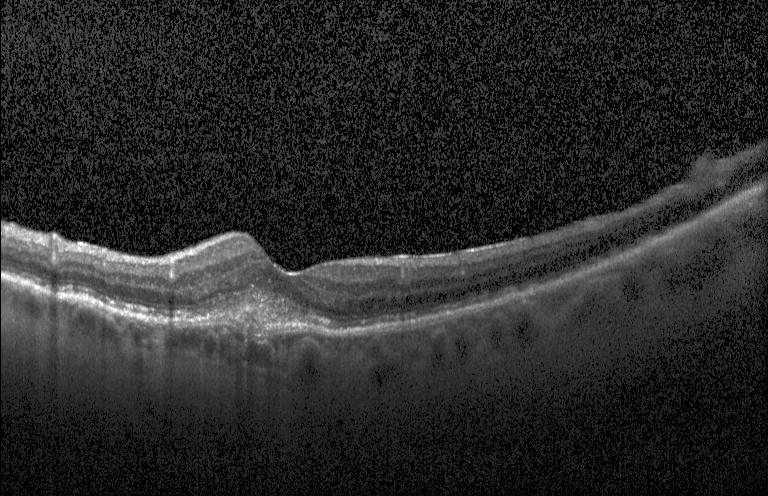 Retinal OCT cross-section showing a choroidal neovascular membrane.